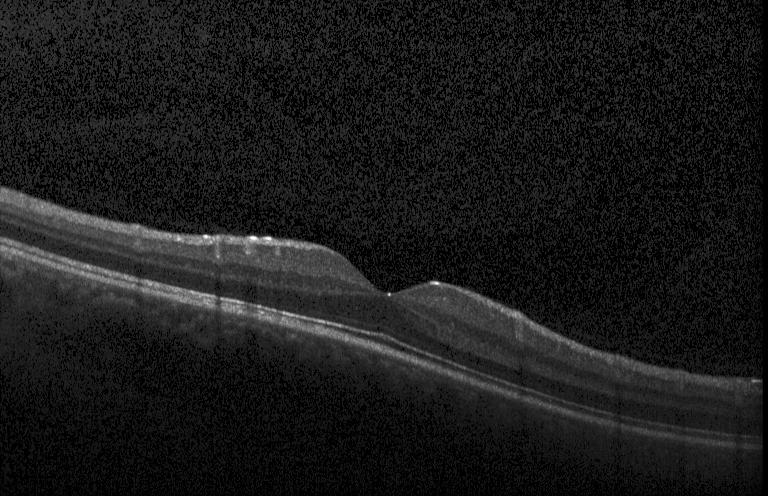 SD-OCT · optical coherence tomography B-scan · fovea-centered — Impression: no evidence of CNV, DME, or drusen.